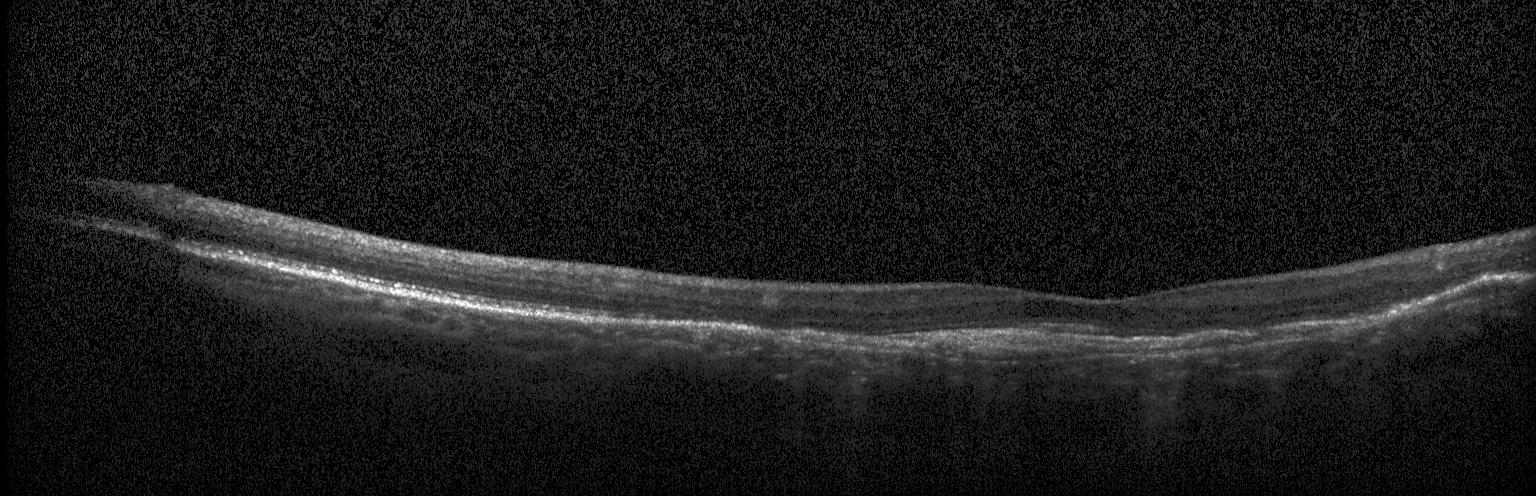
Instrument: Heidelberg Spectralis · horizontal scan through the fovea · retinal OCT B-scan · spectral-domain OCT — Impression: a choroidal neovascular membrane.